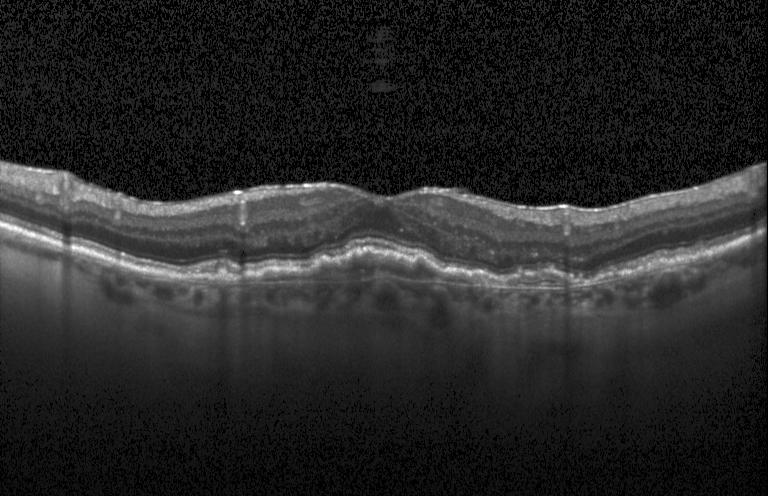 OCT B-scan — Macular OCT: choroidal neovascularization (CNV).